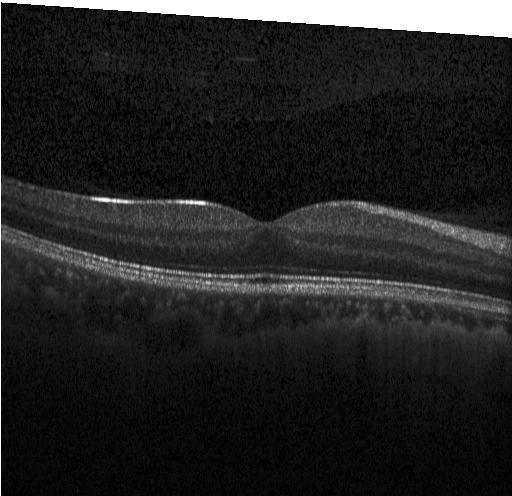
SD-OCT · through the macula · instrument: Heidelberg Spectralis · retinal OCT B-scan — This B-scan demonstrates neither choroidal neovascularization, diabetic macular edema, nor drusen.